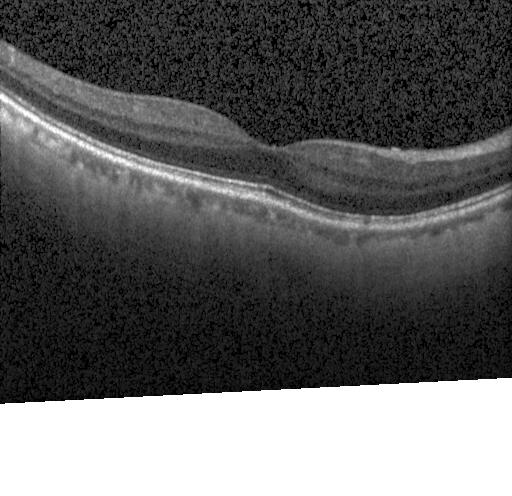 Retinal OCT cross-section; fovea-centered; SD-OCT — Dx: no CNV, DME, or drusen.